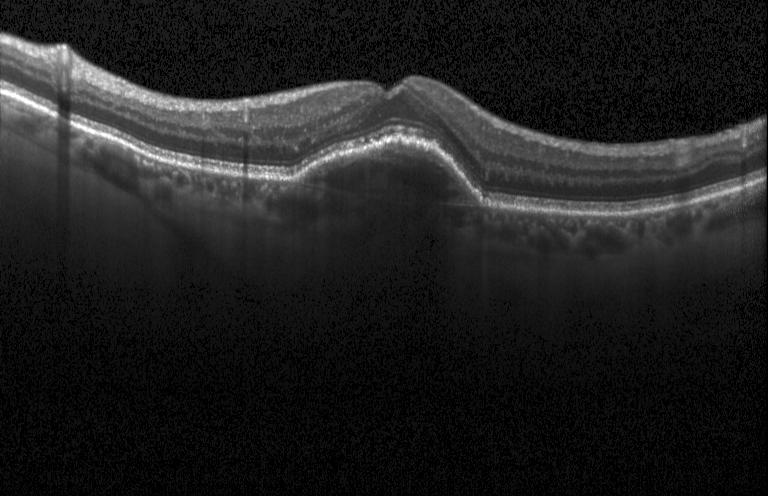
This B-scan demonstrates choroidal neovascularization.